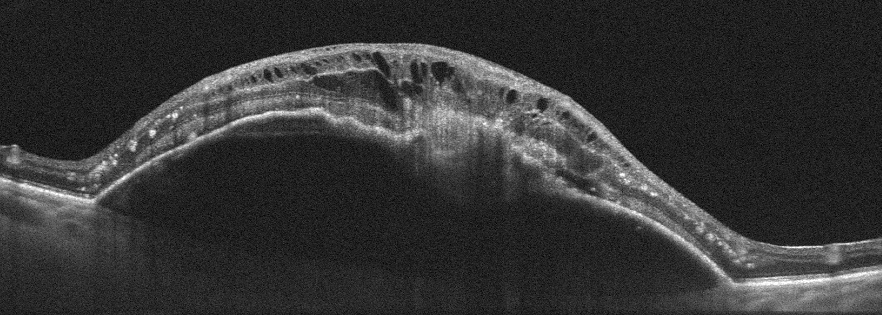 Diagnosis: age-related macular degeneration (AMD).